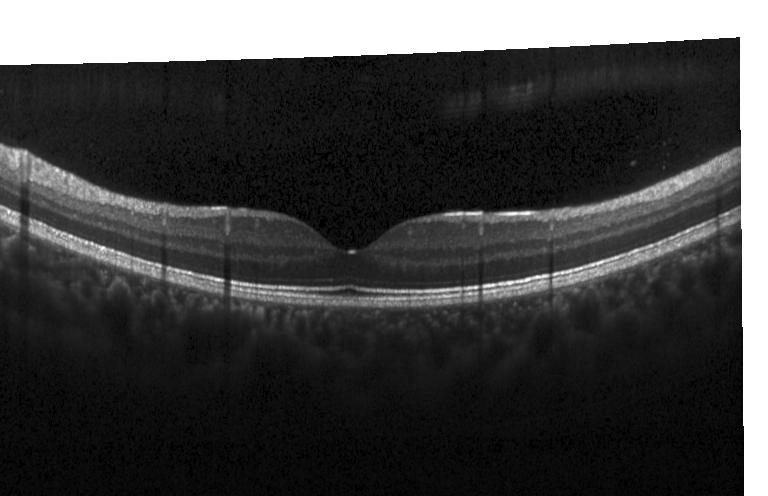 Diagnosis: no evidence of choroidal neovascularization, diabetic macular edema, or drusen.